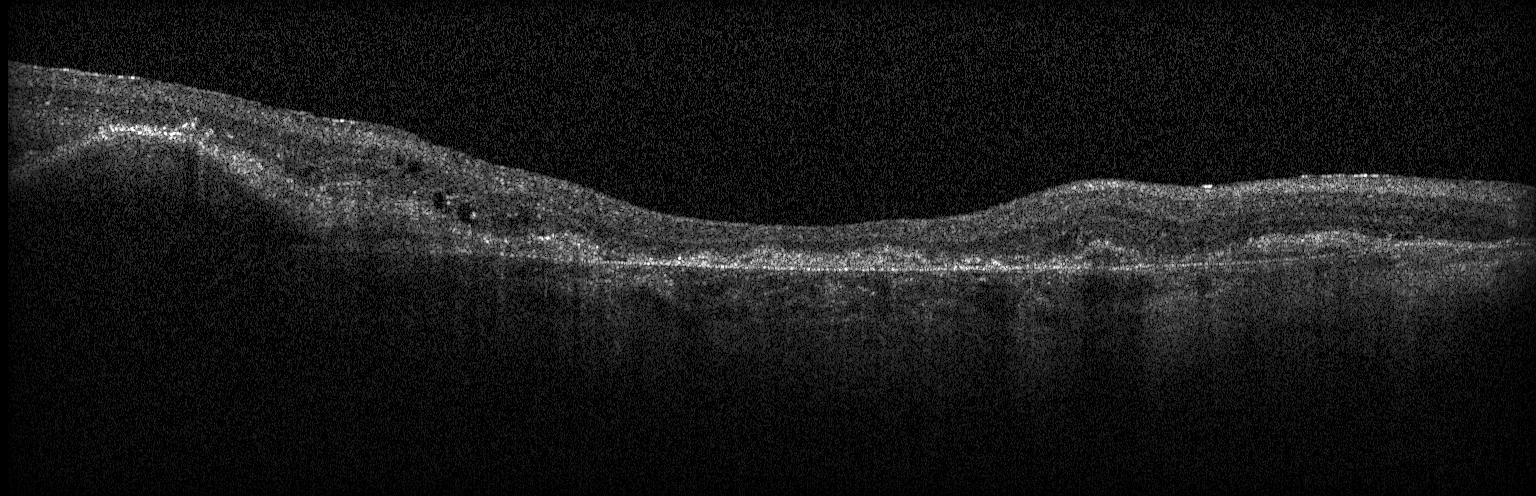

OCT finding: a choroidal neovascular membrane.